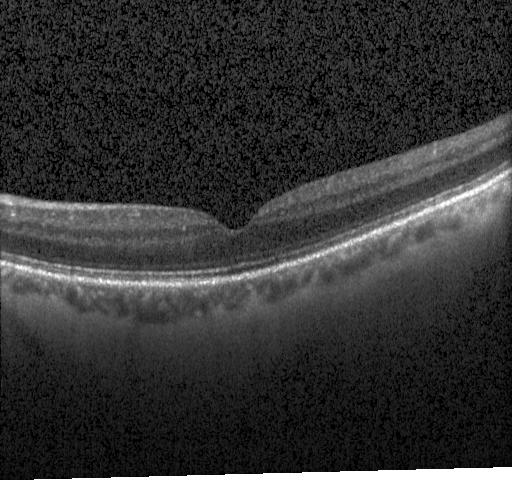

OCT line scan. Horizontal scan through the fovea — Diagnosis: no evidence of CNV, DME, or drusen.